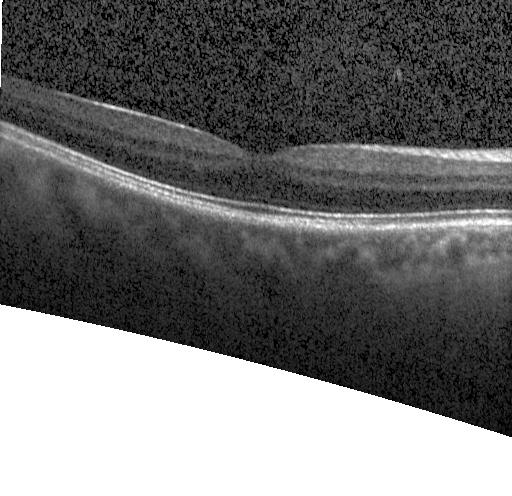

Optical coherence tomography scan. Diagnosis: no CNV, DME, or drusen.